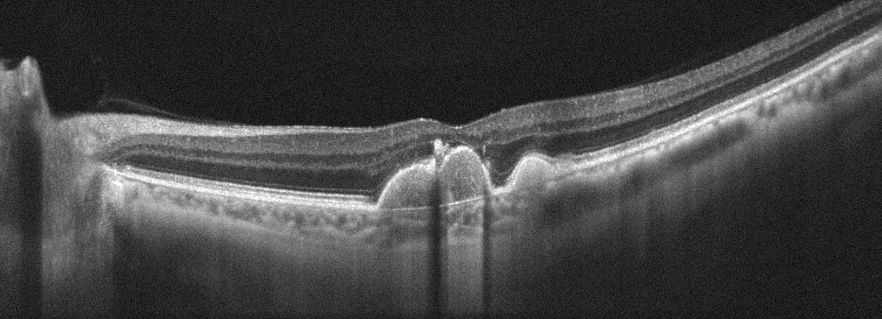
Optical coherence tomography scan; oculus sinister; acquired on an Optovue Avanti RTVue XR.
AMD.